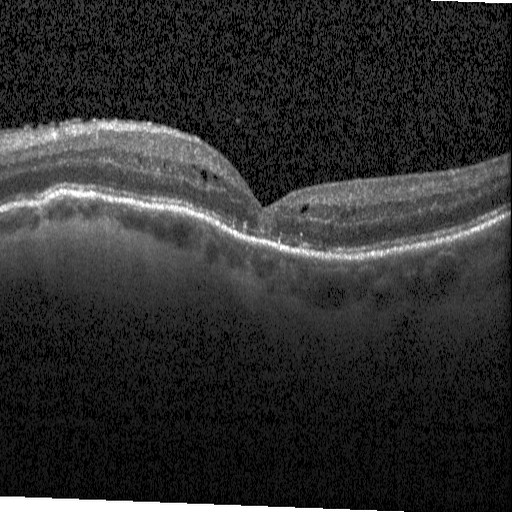
Macular OCT: DME.